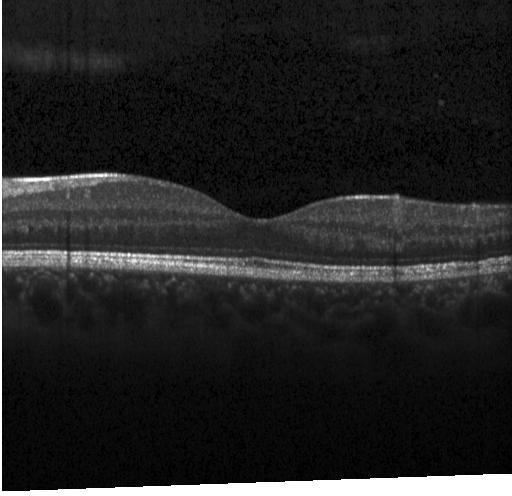
Diagnosis: neither choroidal neovascularization, diabetic macular edema, nor drusen.